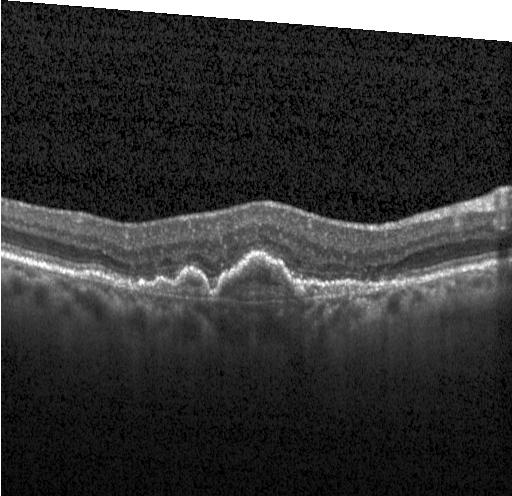
The scan shows choroidal neovascularization (CNV).